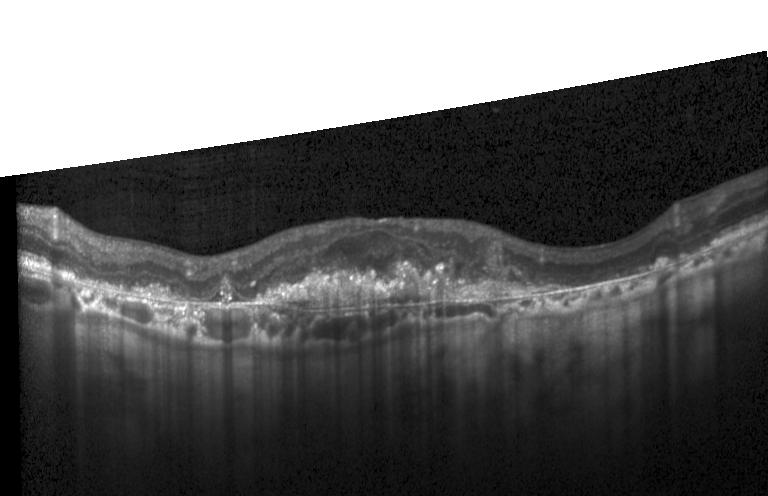
OCT finding: choroidal neovascularization (CNV).